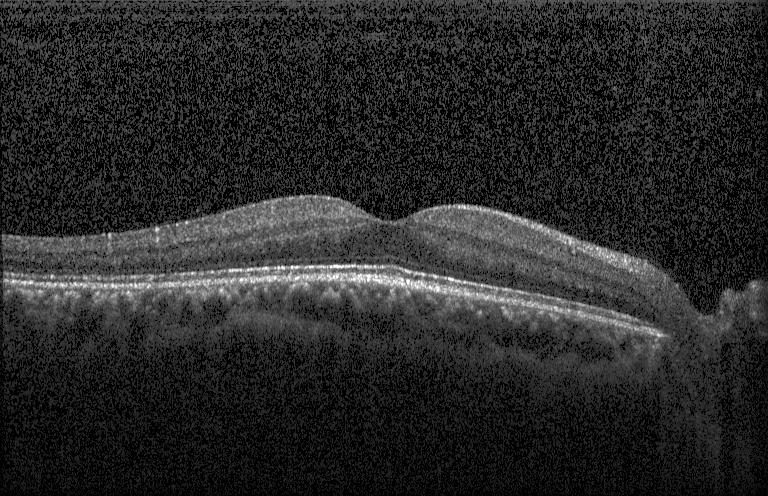 Optical coherence tomography B-scan
Diagnosis: no evidence of CNV, DME, or drusen.